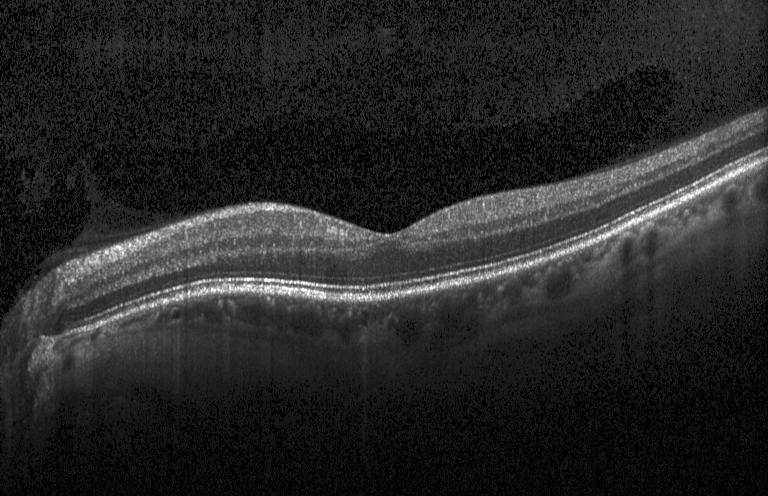 Assessment: no choroidal neovascularization, no diabetic macular edema, and no drusen.